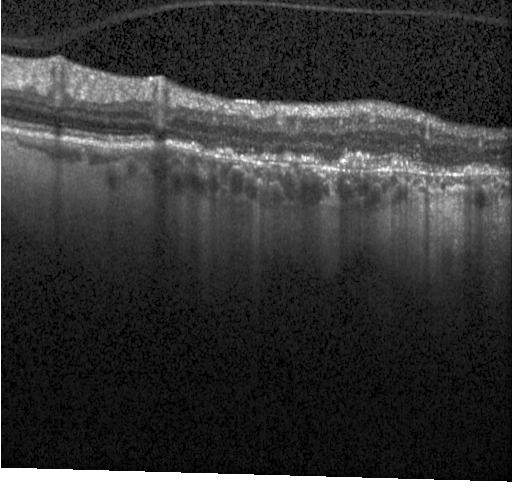
SD-OCT, retinal OCT B-scan, horizontal scan through the fovea.
Assessment: choroidal neovascularization.